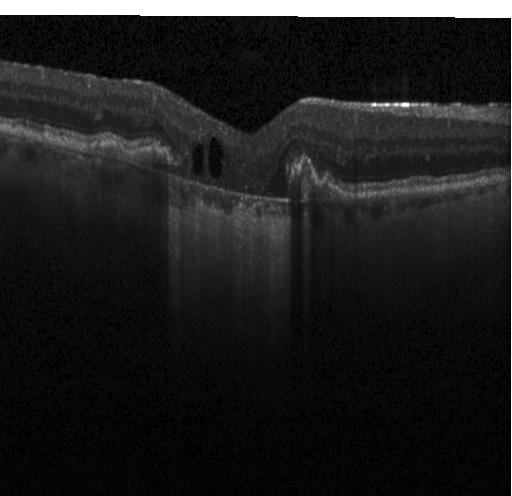 Diagnosis: a choroidal neovascular membrane.